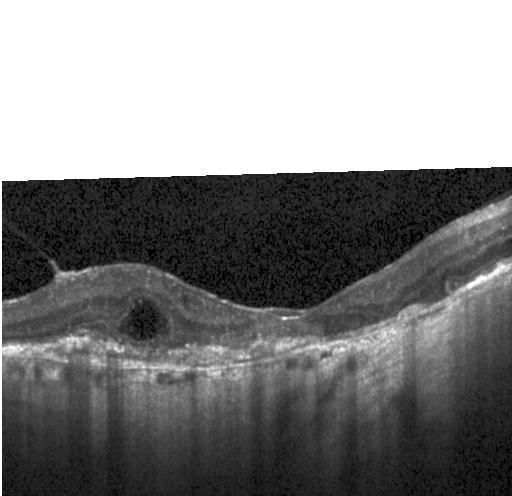
Dx: a choroidal neovascular membrane.